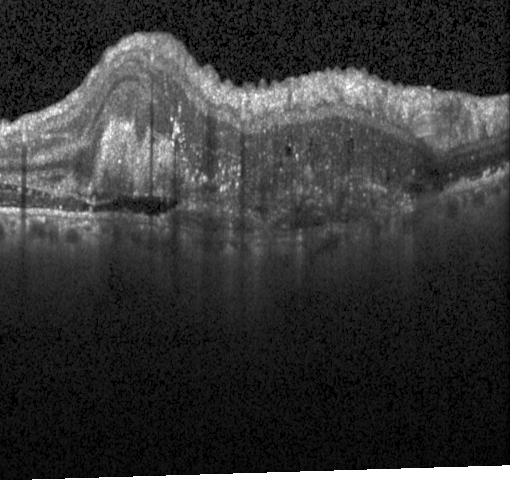

Diagnosis: a choroidal neovascular membrane.